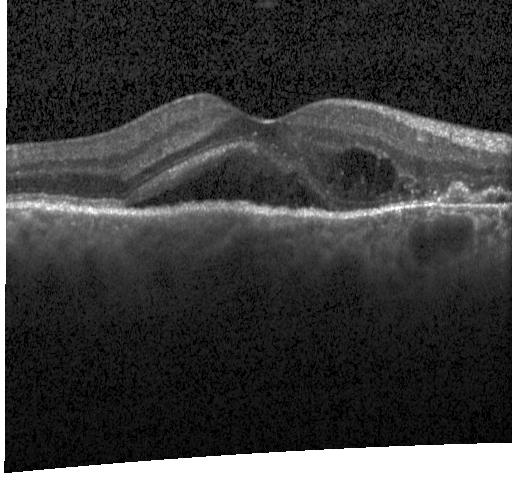 Spectral-domain OCT, fovea-centered, optical coherence tomography B-scan, acquired on a Heidelberg Spectralis.
Finding: choroidal neovascularization (CNV).